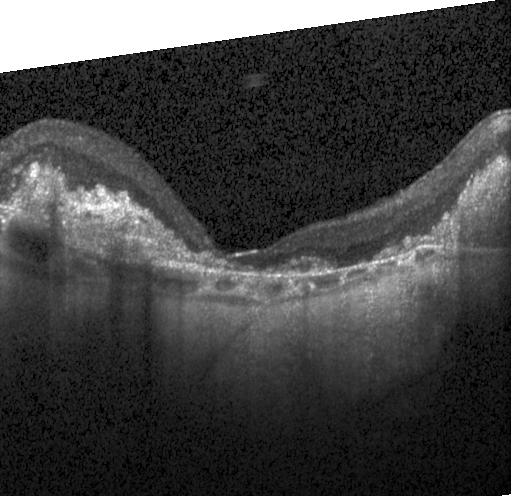 Through the macula, optical coherence tomography B-scan, SD-OCT, acquired on a Heidelberg Spectralis.
Diagnosis: choroidal neovascularization.